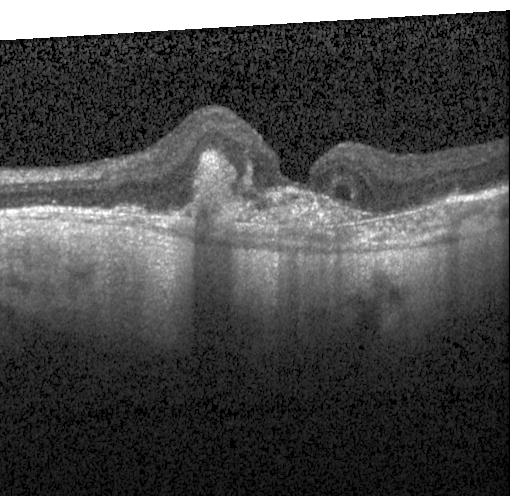 OCT line scan, instrument: Heidelberg Spectralis — Diagnosis: a choroidal neovascular membrane.